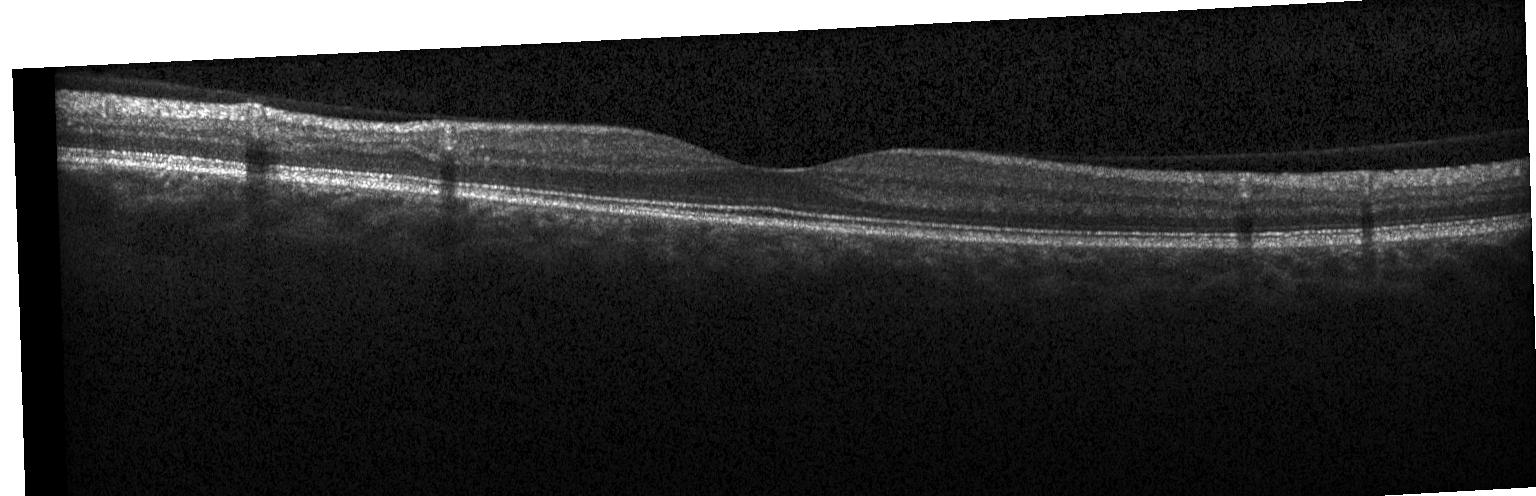 Spectral-domain OCT; retinal OCT cross-section
Diagnosis: no evidence of choroidal neovascularization, diabetic macular edema, or drusen.